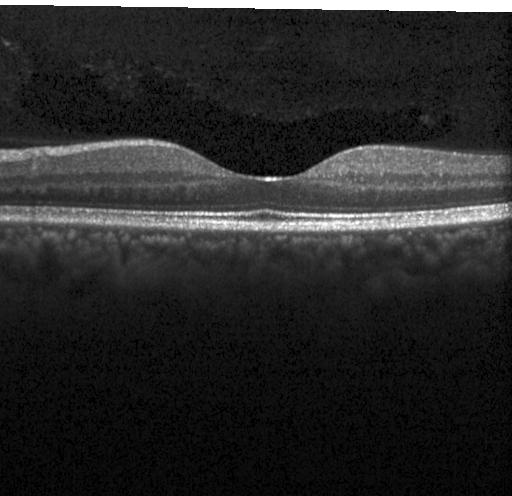
Retinal OCT B-scan.
Finding: no evidence of CNV, DME, or drusen.